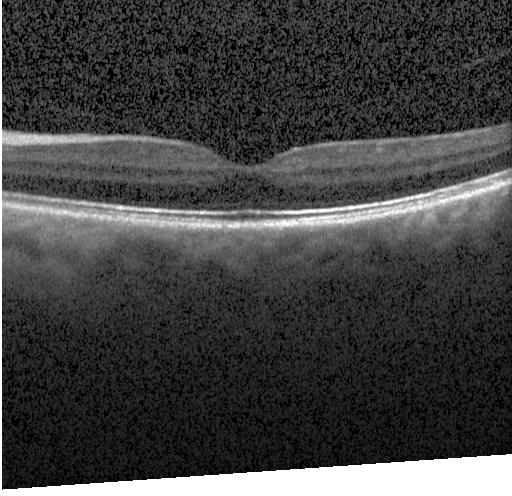
Fovea-centered. OCT line scan.
The scan shows no choroidal neovascularization, no diabetic macular edema, and no drusen.